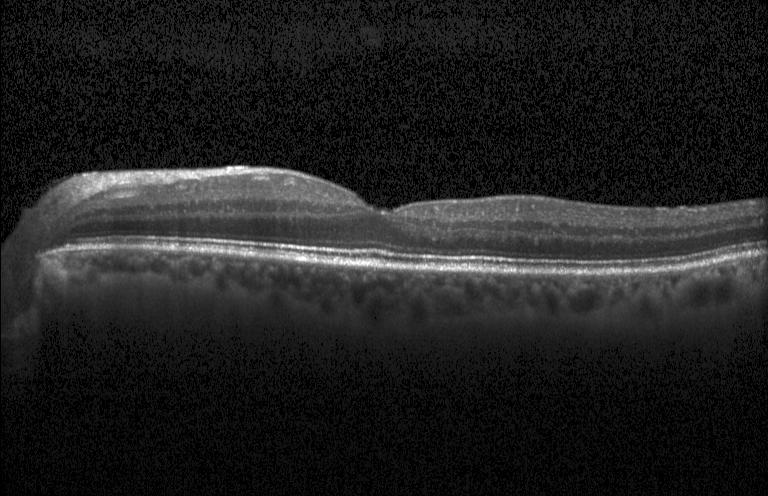
OCT B-scan; instrument: Heidelberg Spectralis. OCT finding: no choroidal neovascularization, diabetic macular edema, or drusen.